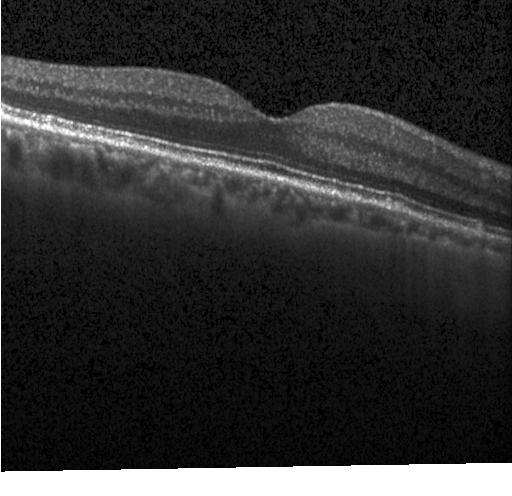 Spectral-domain OCT · acquired on a Heidelberg Spectralis · through the macula · optical coherence tomography scan. Diagnosis: no choroidal neovascularization, diabetic macular edema, or drusen.